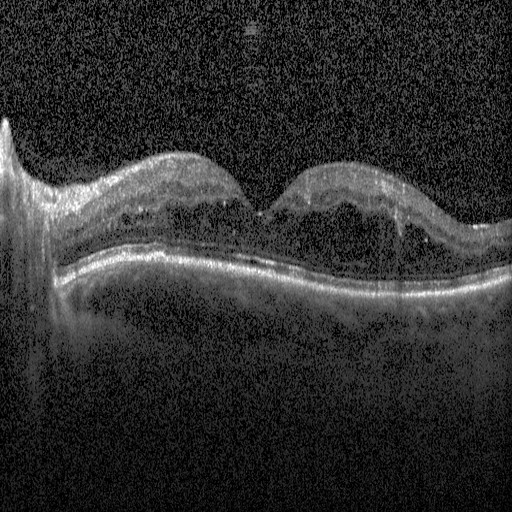

OCT B-scan showing diabetic macular edema.